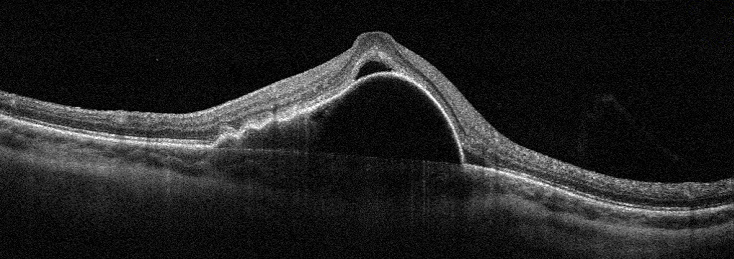
AMD.